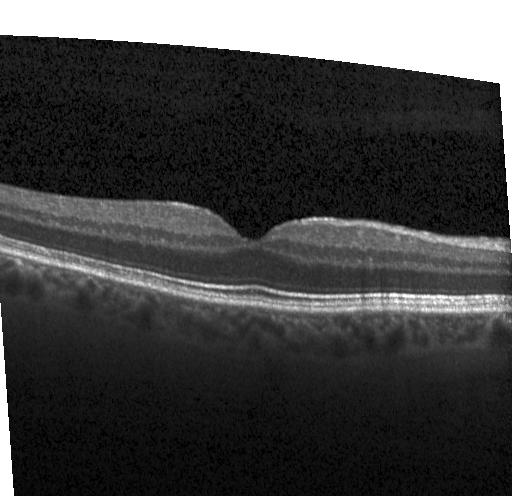
Heidelberg Spectralis, optical coherence tomography B-scan.
Impression: no choroidal neovascularization, no diabetic macular edema, and no drusen.